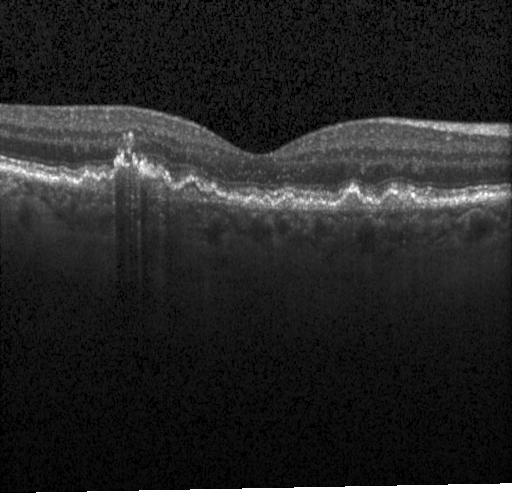 OCT line scan · instrument: Heidelberg Spectralis
Impression: choroidal neovascularization (CNV).